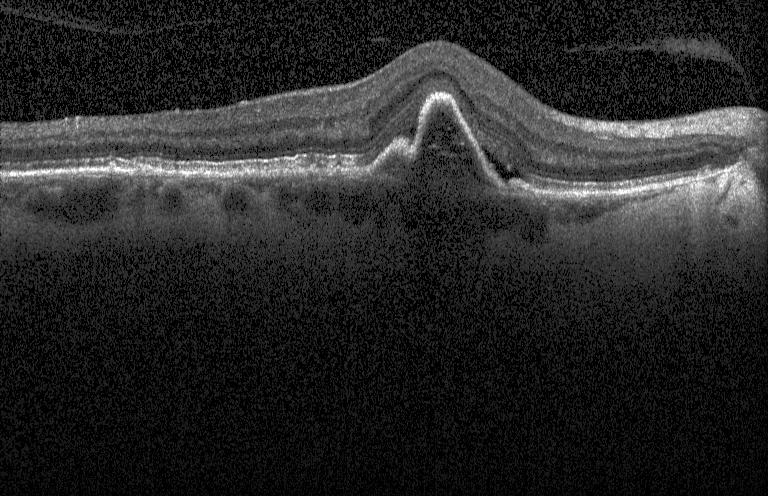 Macular scan, optical coherence tomography B-scan.
Diagnosis: a choroidal neovascular membrane.